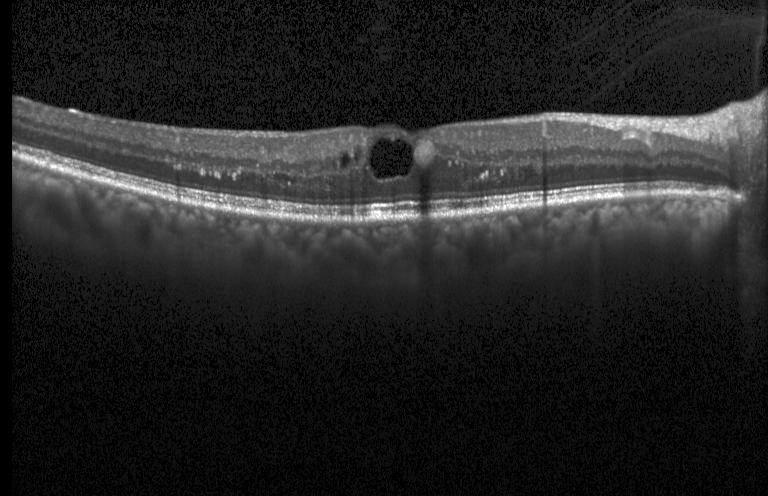

Dx: diabetic macular edema (DME).